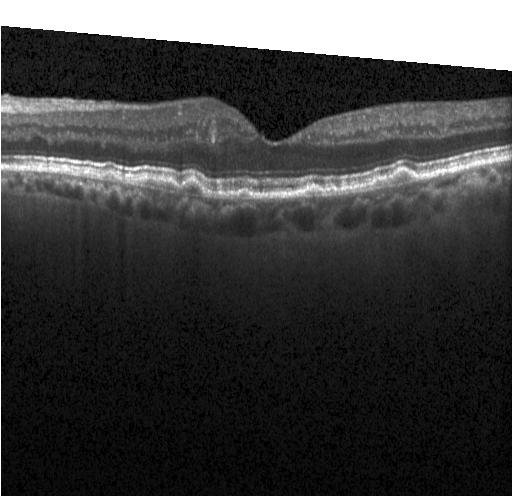 Through the macula. Spectral-domain OCT. Optical coherence tomography scan. Heidelberg Spectralis
This B-scan demonstrates drusen.